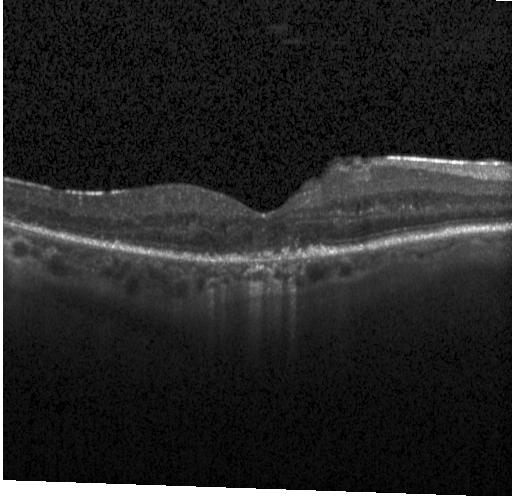 Spectral-domain optical coherence tomography. Heidelberg Spectralis OCT system. Retinal OCT B-scan. The scan shows no evidence of choroidal neovascularization, diabetic macular edema, or drusen.